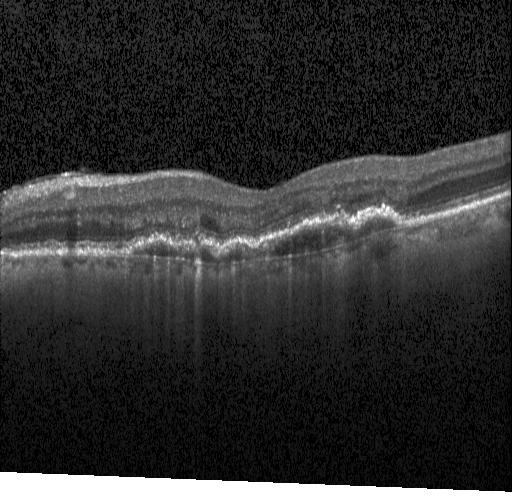 Retinal OCT B-scan.
Diagnosis: a choroidal neovascular membrane.